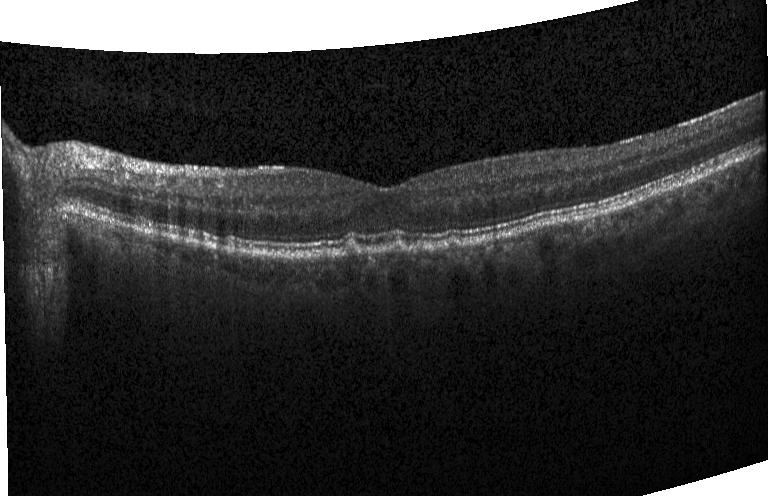

OCT finding: sub-RPE drusenoid deposits.